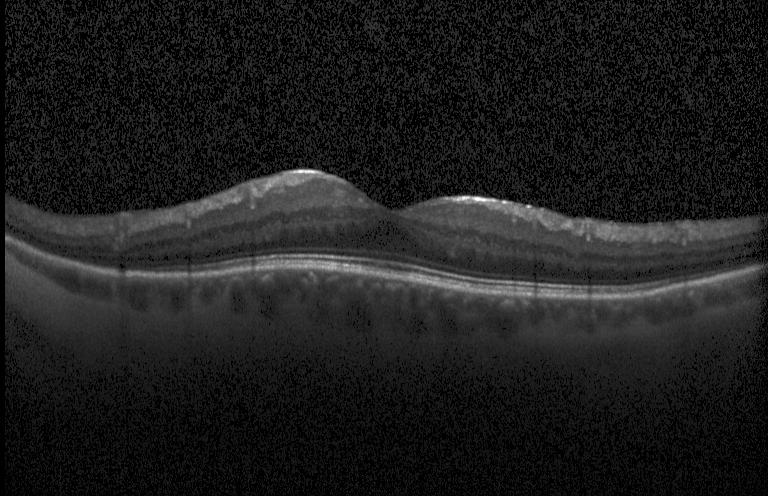 Optical coherence tomography scan · Heidelberg Spectralis — Diagnosis: no evidence of CNV, DME, or drusen.